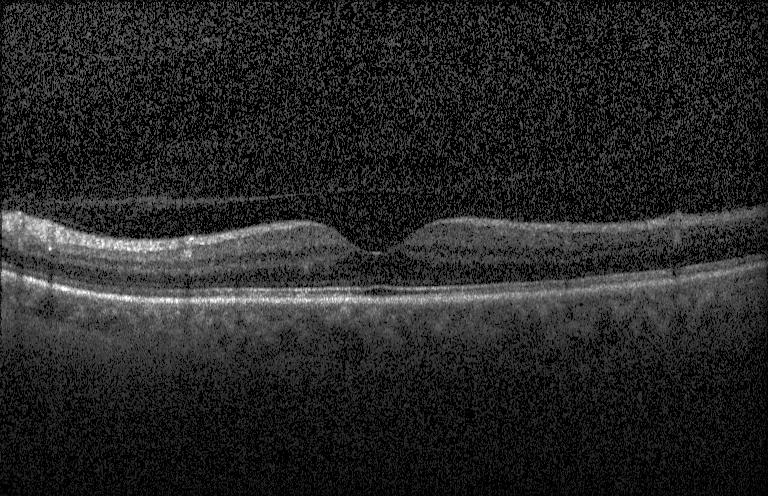

Acquired on a Heidelberg Spectralis · spectral-domain optical coherence tomography · optical coherence tomography scan — The scan shows neither CNV, DME, nor drusen.